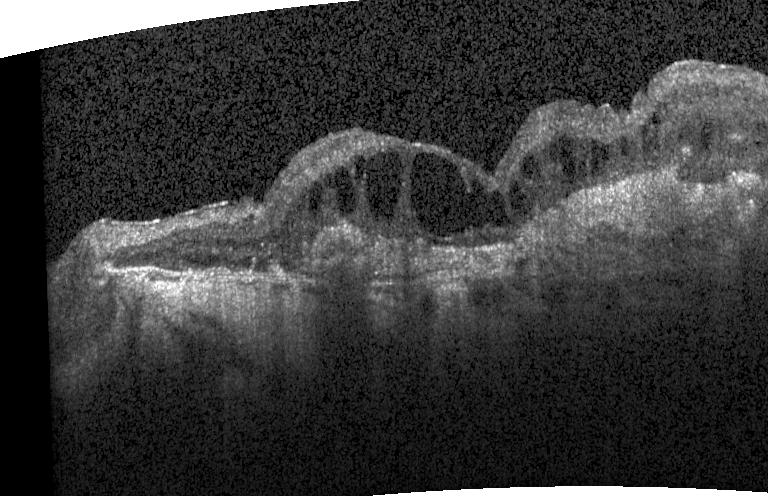 OCT line scan — Finding: choroidal neovascularization (CNV).